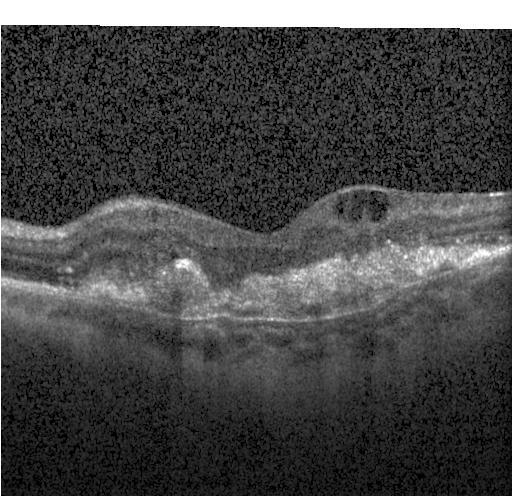
Diagnosis: a choroidal neovascular membrane.